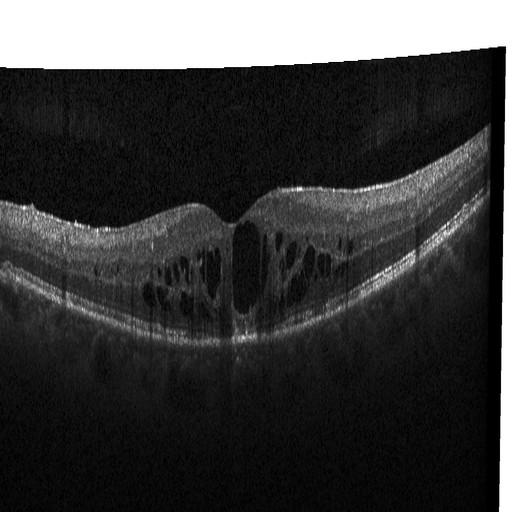 DME.